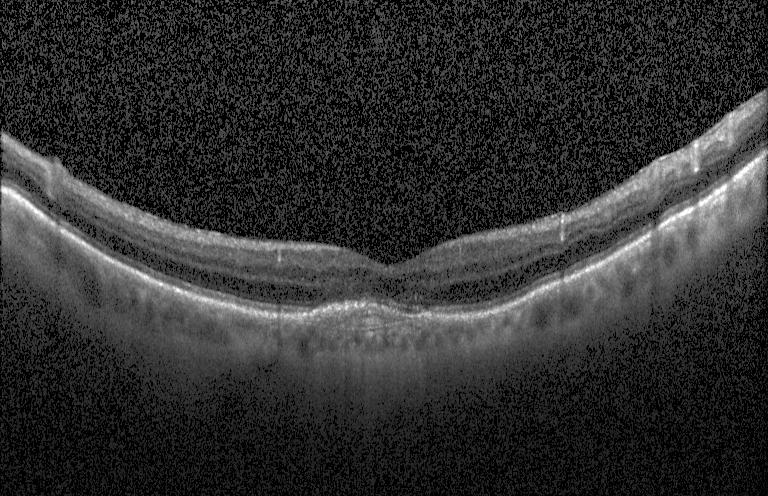
Spectral-domain optical coherence tomography, instrument: Heidelberg Spectralis, through the macula, optical coherence tomography B-scan. OCT finding: choroidal neovascularization.